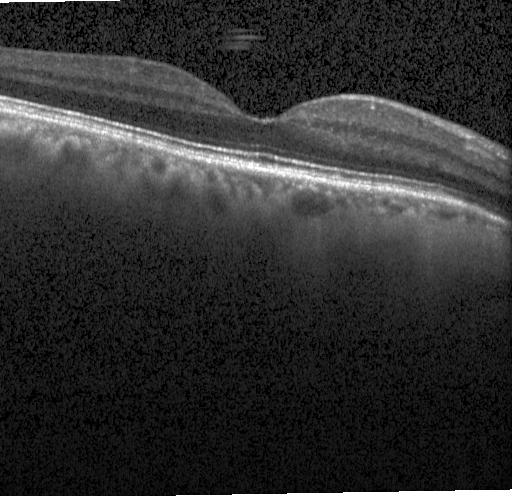
Macular OCT: no CNV, no DME, and no drusen.